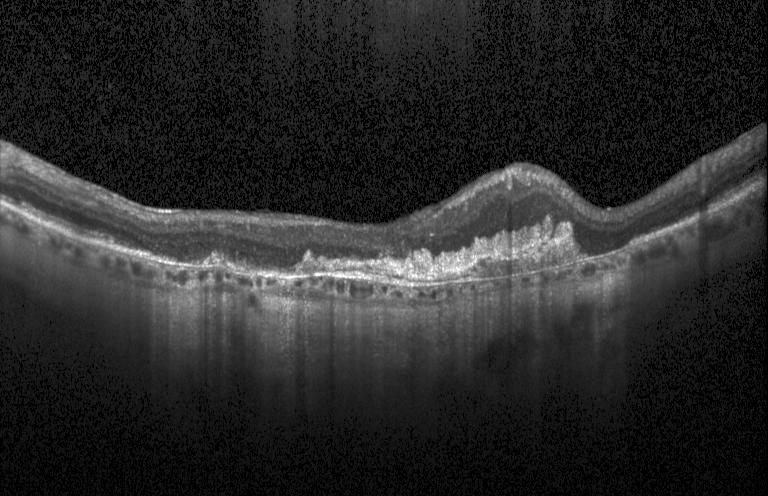 Retinal OCT cross-section. Fovea-centered. Heidelberg Spectralis. Assessment: choroidal neovascularization.